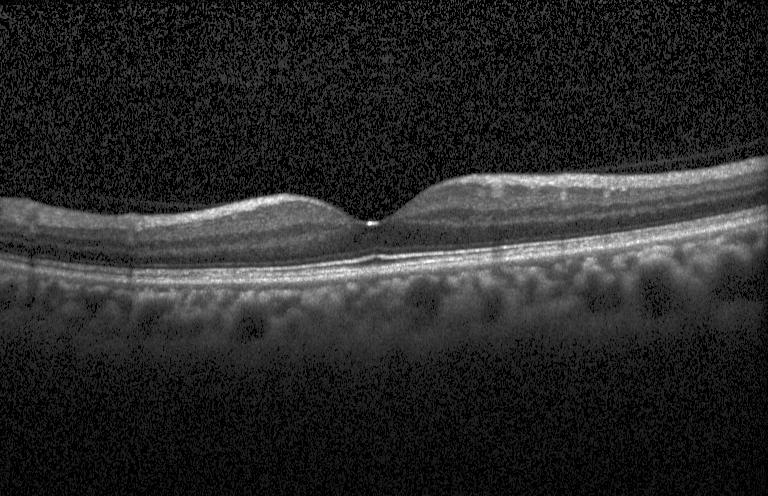
Through the macula; optical coherence tomography B-scan; spectral-domain optical coherence tomography; Heidelberg Spectralis OCT system.
Finding: no choroidal neovascularization, no diabetic macular edema, and no drusen.